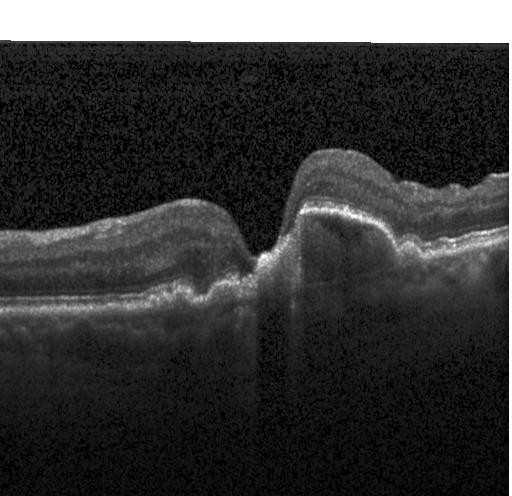

Spectral-domain optical coherence tomography; OCT line scan. The scan shows a choroidal neovascular membrane.